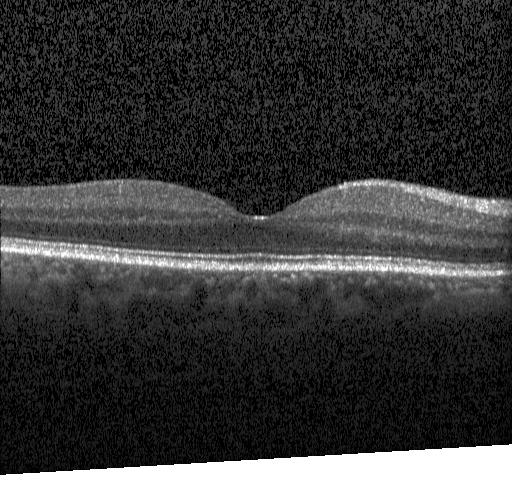
Retinal OCT cross-section
Finding: neither choroidal neovascularization, diabetic macular edema, nor drusen.